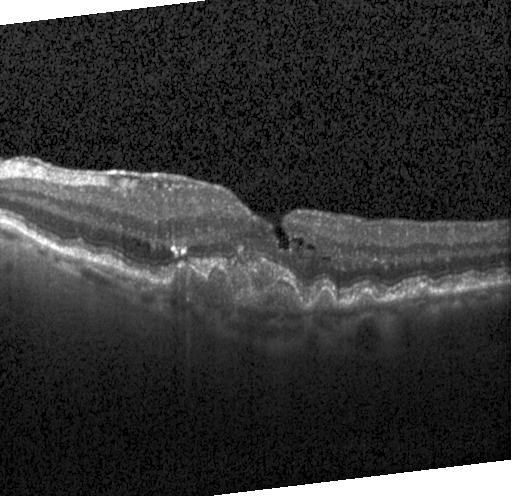

OCT B-scan showing a choroidal neovascular membrane.